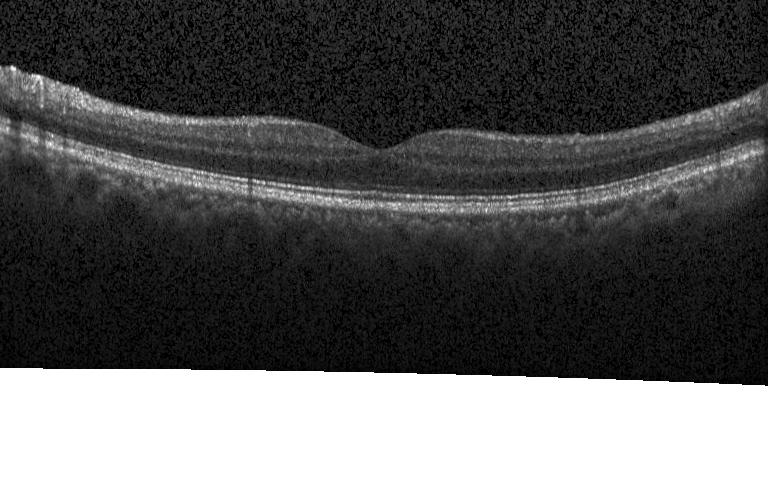

Horizontal scan through the fovea, OCT line scan
Impression: no choroidal neovascularization, no diabetic macular edema, and no drusen.